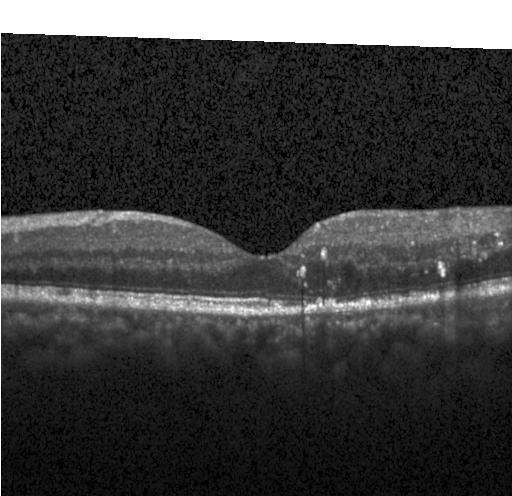

Optical coherence tomography B-scan, spectral-domain optical coherence tomography. Diagnosis: diabetic macular edema.